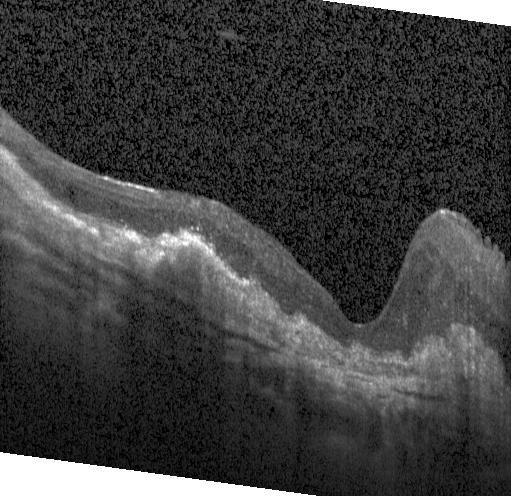
CNV.